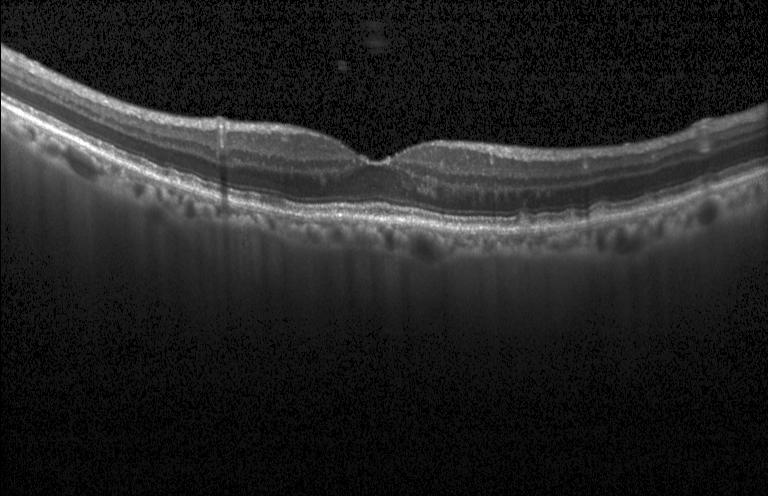

Macular OCT: drusen.